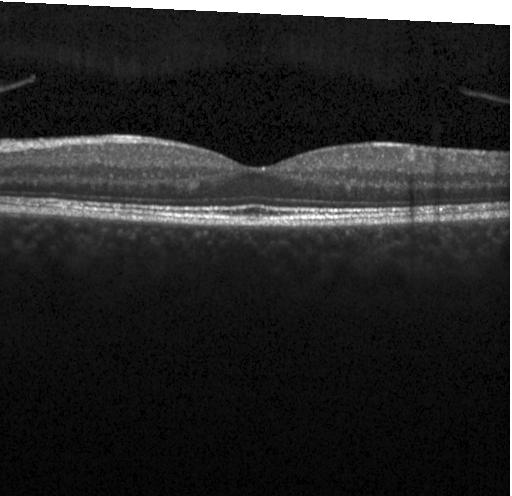

Optical coherence tomography B-scan, SD-OCT, horizontal scan through the fovea, instrument: Heidelberg Spectralis
Impression: no evidence of choroidal neovascularization, diabetic macular edema, or drusen.